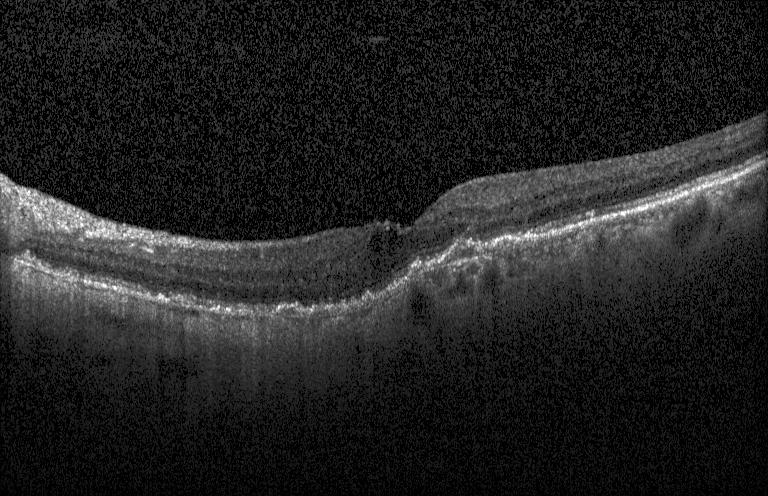 Spectral-domain optical coherence tomography · instrument: Heidelberg Spectralis · macular scan · retinal OCT B-scan
Assessment: a choroidal neovascular membrane.